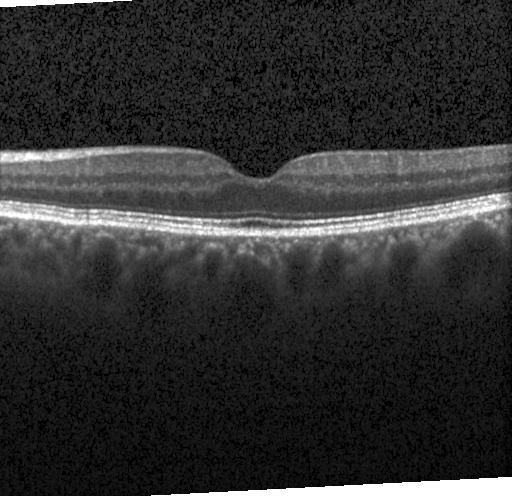

Spectral-domain optical coherence tomography; retinal OCT B-scan. No evidence of choroidal neovascularization, diabetic macular edema, or drusen.